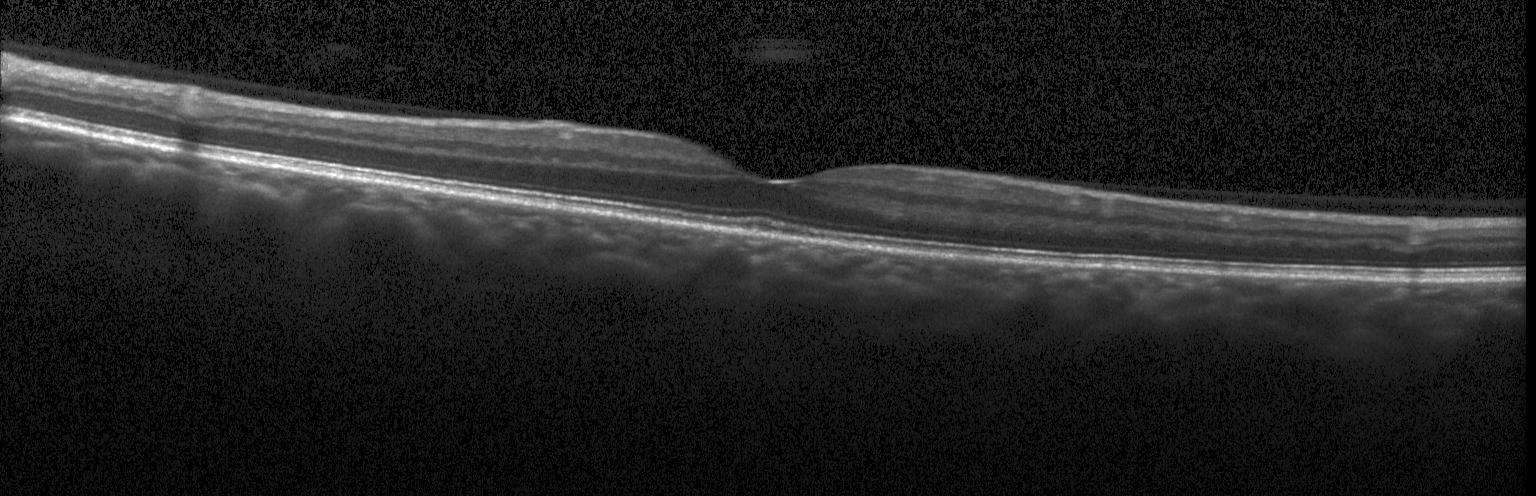

Acquired on a Heidelberg Spectralis · horizontal scan through the fovea · optical coherence tomography B-scan. No evidence of CNV, DME, or drusen.